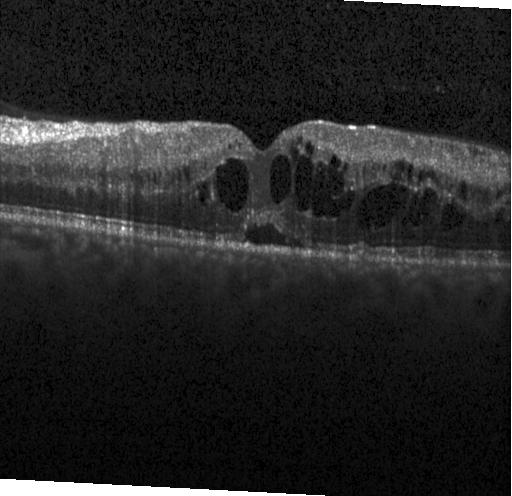 Optical coherence tomography B-scan — Diabetic macular edema.